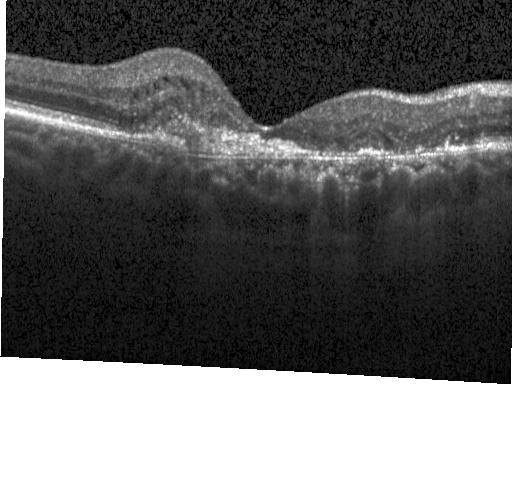
Spectral-domain optical coherence tomography; OCT B-scan. Diagnosis: a choroidal neovascular membrane.